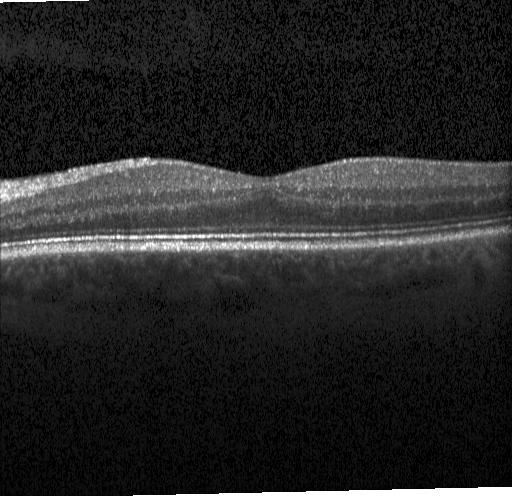
Impression: no CNV, DME, or drusen.